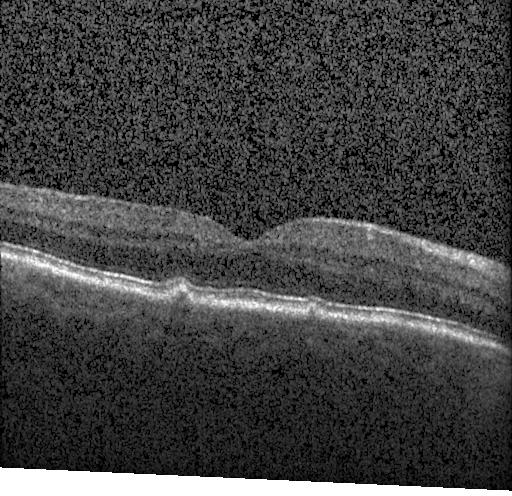
Macular scan; acquired on a Heidelberg Spectralis; optical coherence tomography scan.
Finding: sub-RPE drusenoid deposits.